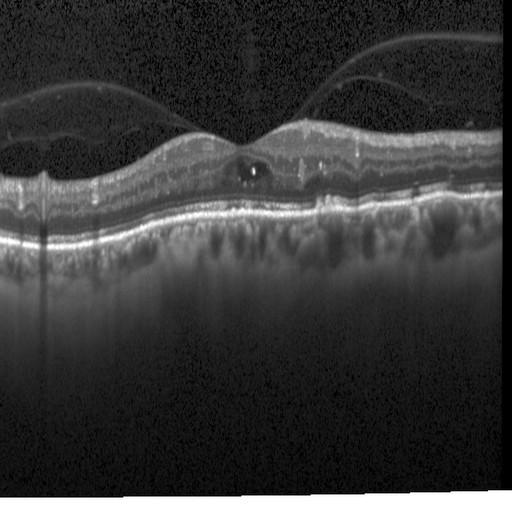
Spectral-domain OCT, centered on the fovea, retinal OCT B-scan — This B-scan demonstrates diabetic macular edema (DME).